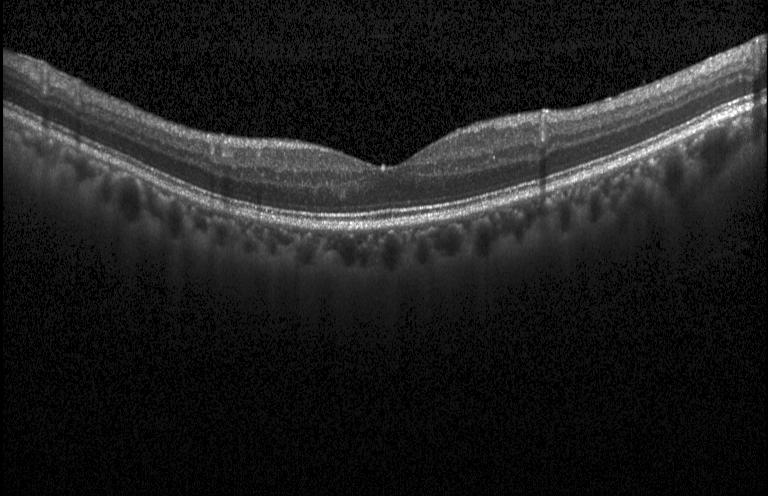 OCT line scan. SD-OCT. Instrument: Heidelberg Spectralis. Fovea-centered.
Macular OCT: no evidence of CNV, DME, or drusen.